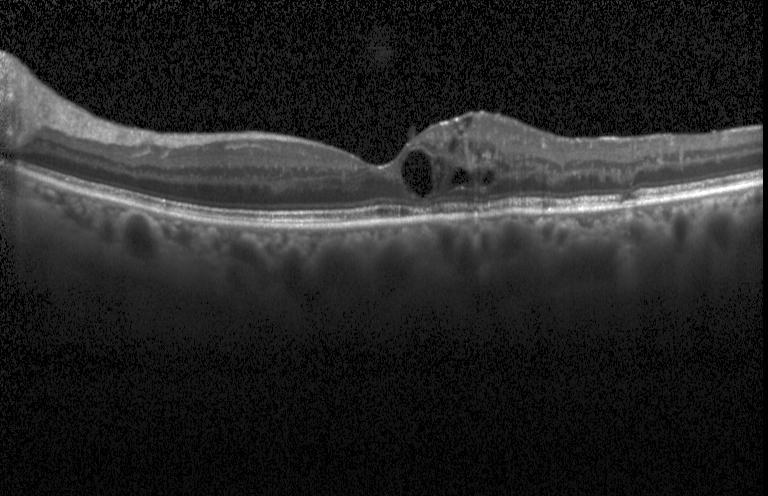 OCT B-scan, centered on the fovea, Heidelberg Spectralis, spectral-domain optical coherence tomography — Diagnosis: diabetic macular edema (DME).